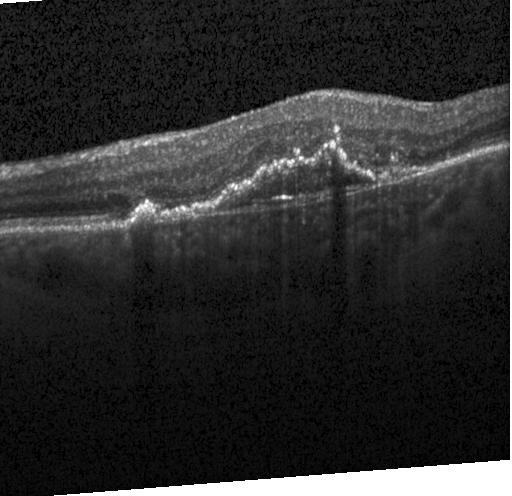 This B-scan demonstrates choroidal neovascularization.